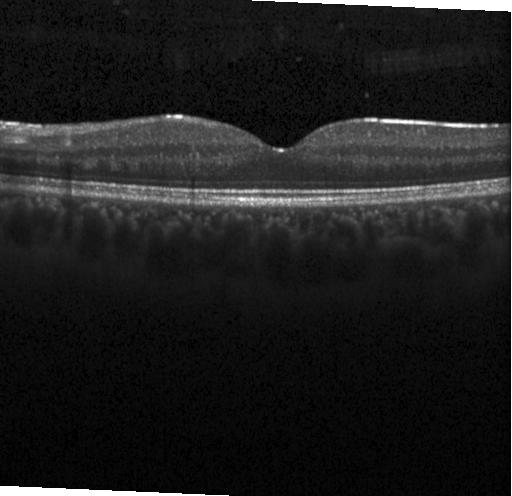
OCT scan showing no evidence of choroidal neovascularization, diabetic macular edema, or drusen.